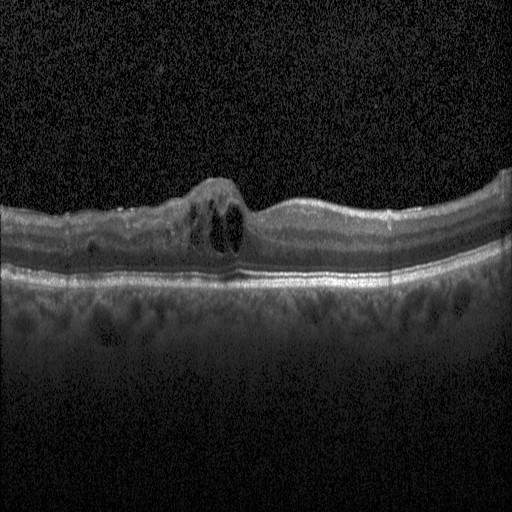
OCT B-scan. Centered on the fovea
OCT finding: diabetic macular edema (DME).